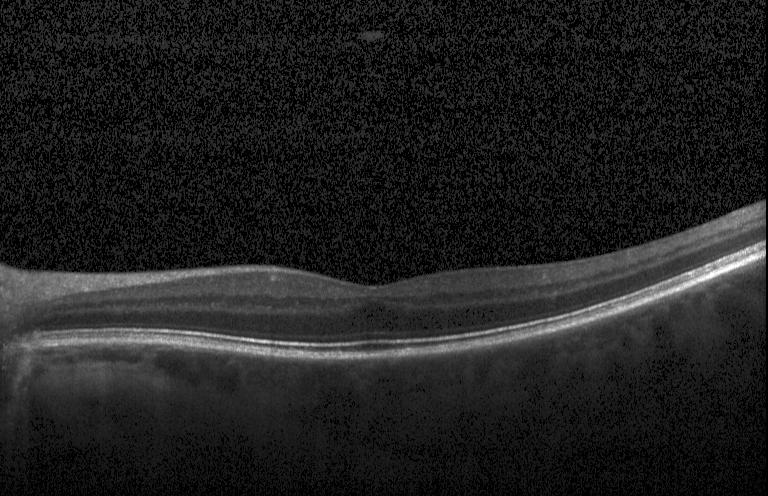 Optical coherence tomography scan
Impression: no CNV, DME, or drusen.